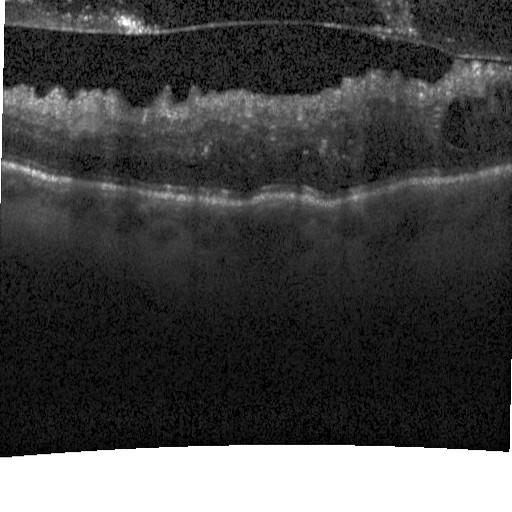

OCT B-scan showing diabetic macular edema.